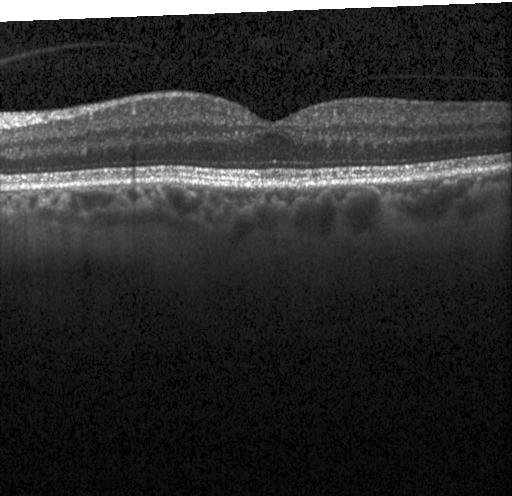
Optical coherence tomography scan — Impression: no CNV, no DME, and no drusen.